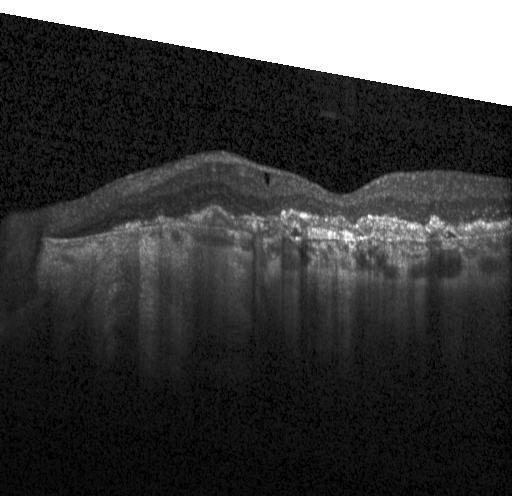
Optical coherence tomography B-scan. SD-OCT — Diagnosis: a choroidal neovascular membrane.